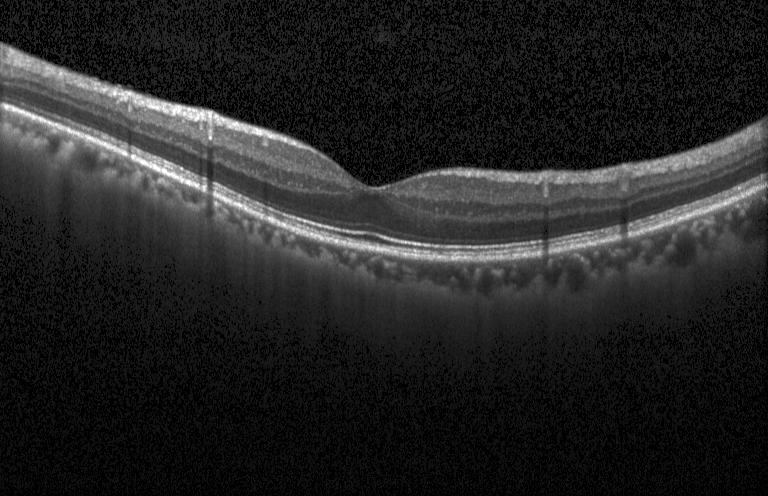

Spectral-domain OCT B-scan: no choroidal neovascularization, diabetic macular edema, or drusen.